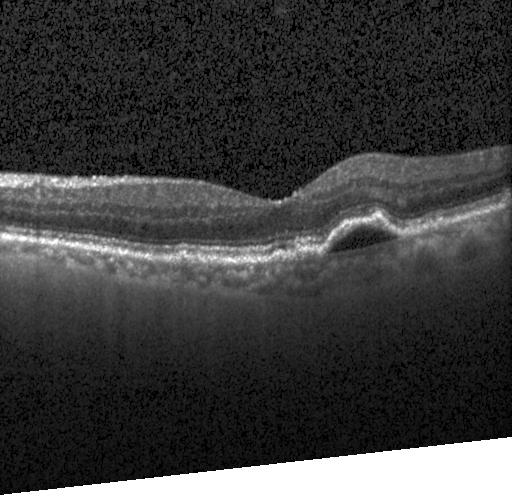

Heidelberg Spectralis OCT system · optical coherence tomography scan · SD-OCT
OCT finding: choroidal neovascularization (CNV).